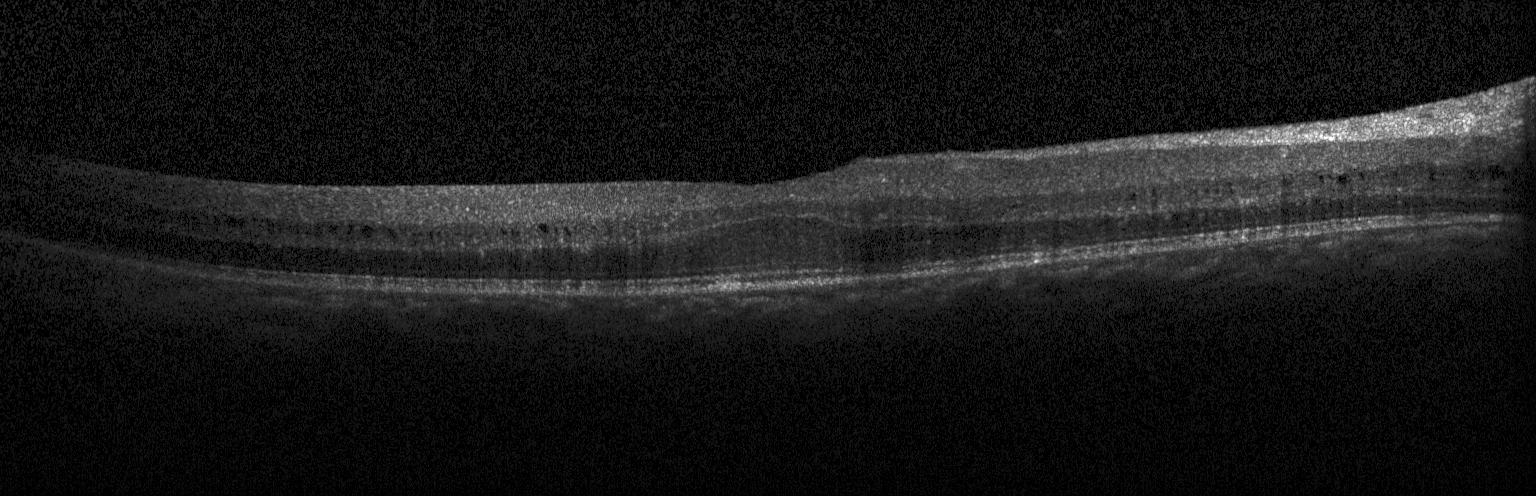
Macular OCT demonstrating diabetic macular edema.